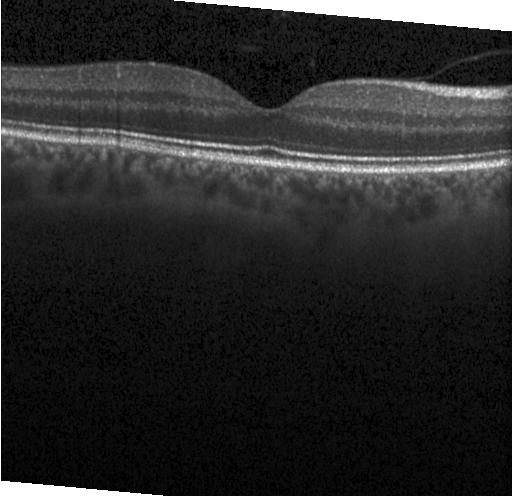

Heidelberg Spectralis, retinal OCT cross-section, centered on the fovea.
OCT finding: no choroidal neovascularization, diabetic macular edema, or drusen.